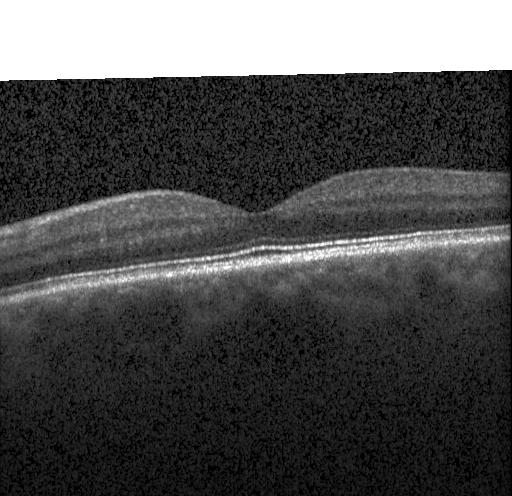

Optical coherence tomography scan.
The scan shows neither choroidal neovascularization, diabetic macular edema, nor drusen.